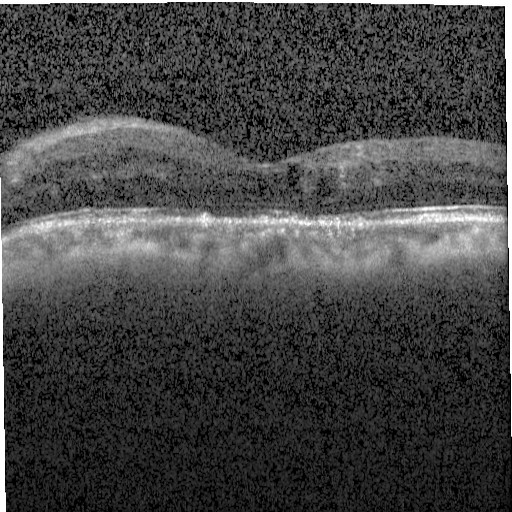
OCT finding: DME.